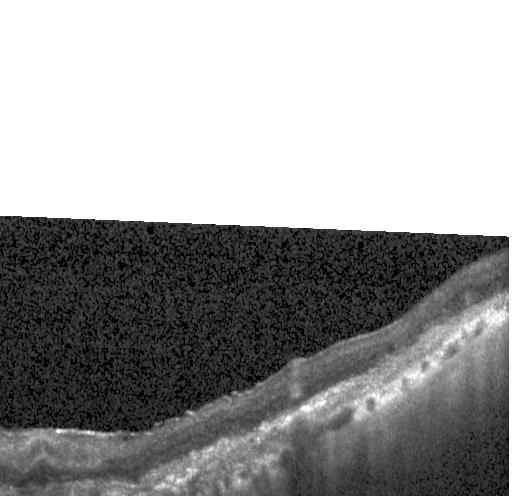

Diagnosis: a choroidal neovascular membrane.